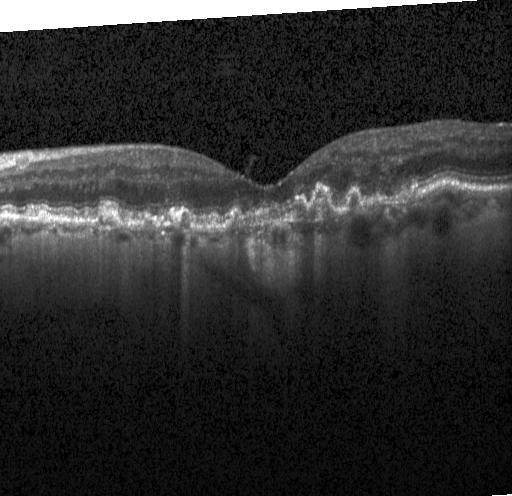 The scan shows drusen.